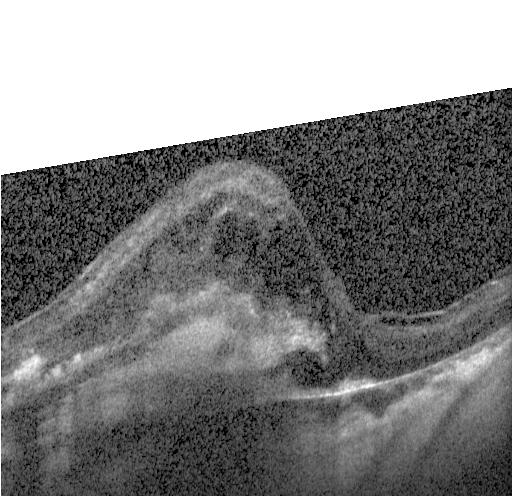
Spectral-domain optical coherence tomography; retinal OCT B-scan.
This B-scan demonstrates a choroidal neovascular membrane.